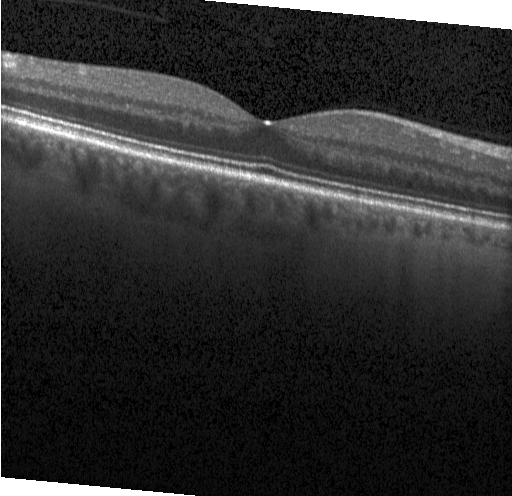
Dx: no choroidal neovascularization, diabetic macular edema, or drusen.